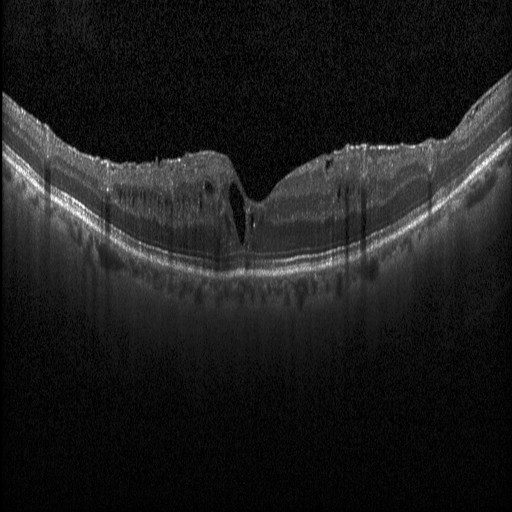
Centered on the fovea; optical coherence tomography B-scan
The scan shows DME.